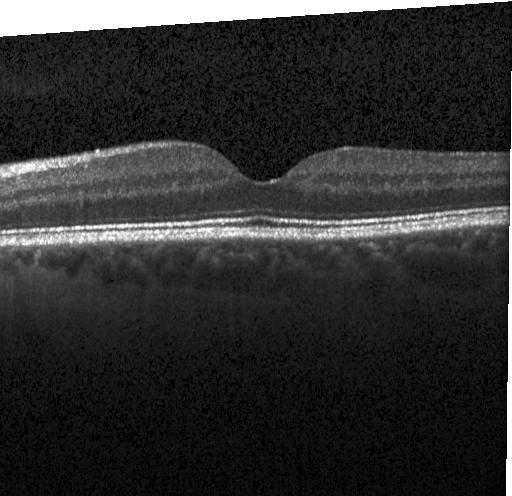

Centered on the fovea, retinal OCT cross-section.
Finding: no evidence of CNV, DME, or drusen.